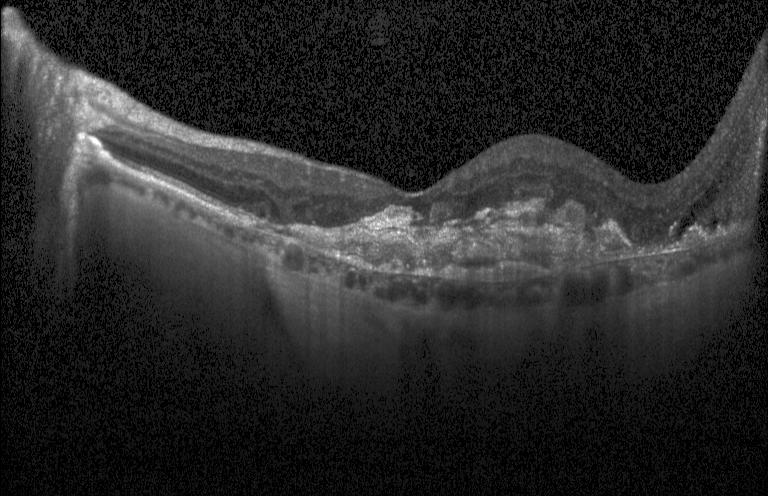
Finding: CNV.